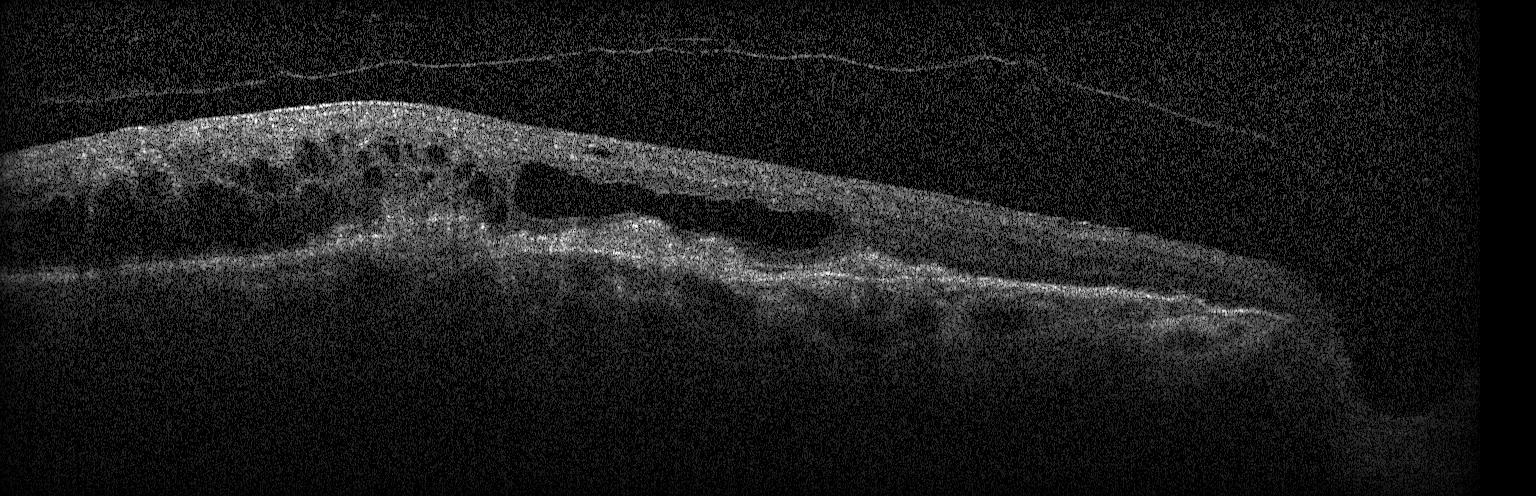

Optical coherence tomography B-scan. Finding: a choroidal neovascular membrane.